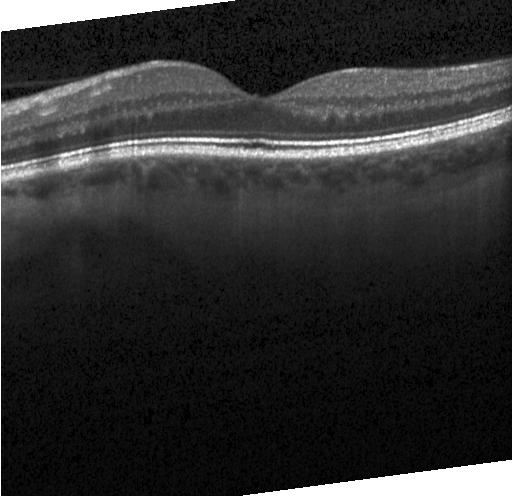
Diagnosis: no evidence of choroidal neovascularization, diabetic macular edema, or drusen.